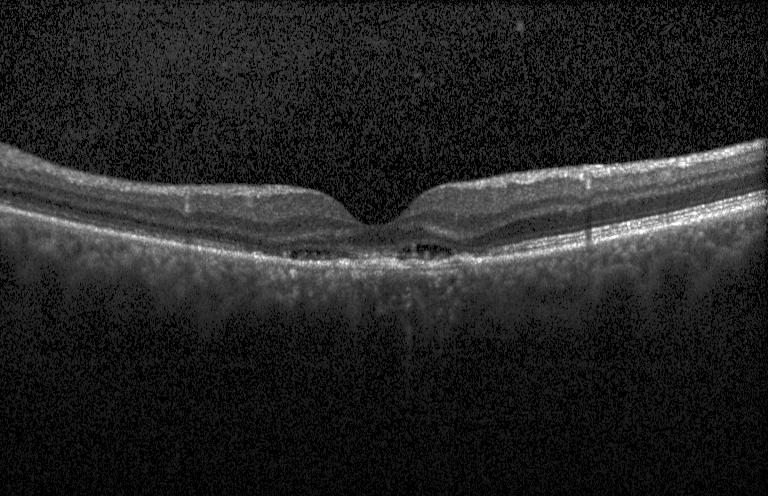 Fovea-centered, acquired on a Heidelberg Spectralis, SD-OCT, optical coherence tomography scan
CNV.